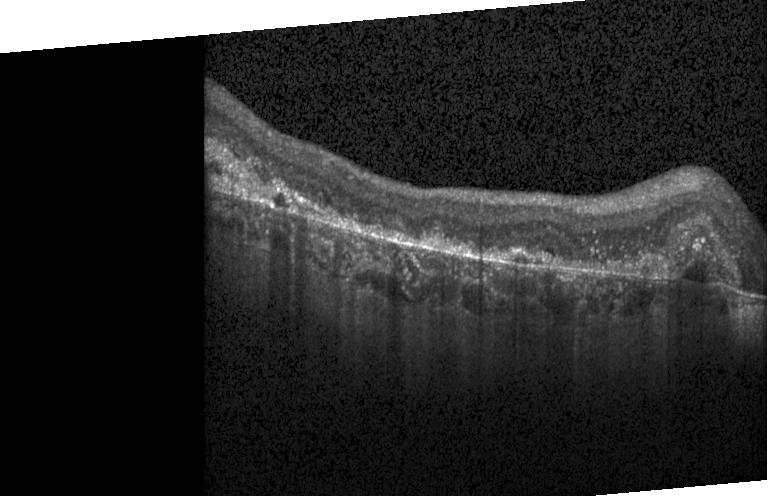

Optical coherence tomography B-scan.
The scan shows CNV.